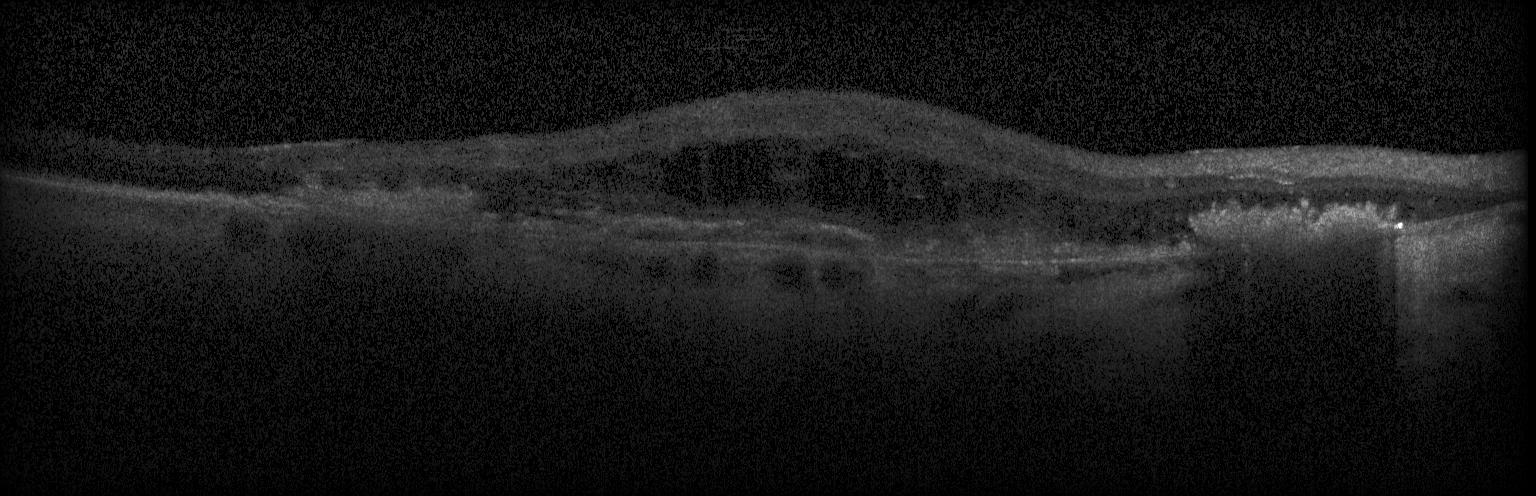
Horizontal scan through the fovea · acquired on a Heidelberg Spectralis · optical coherence tomography B-scan · spectral-domain OCT. Finding: CNV.